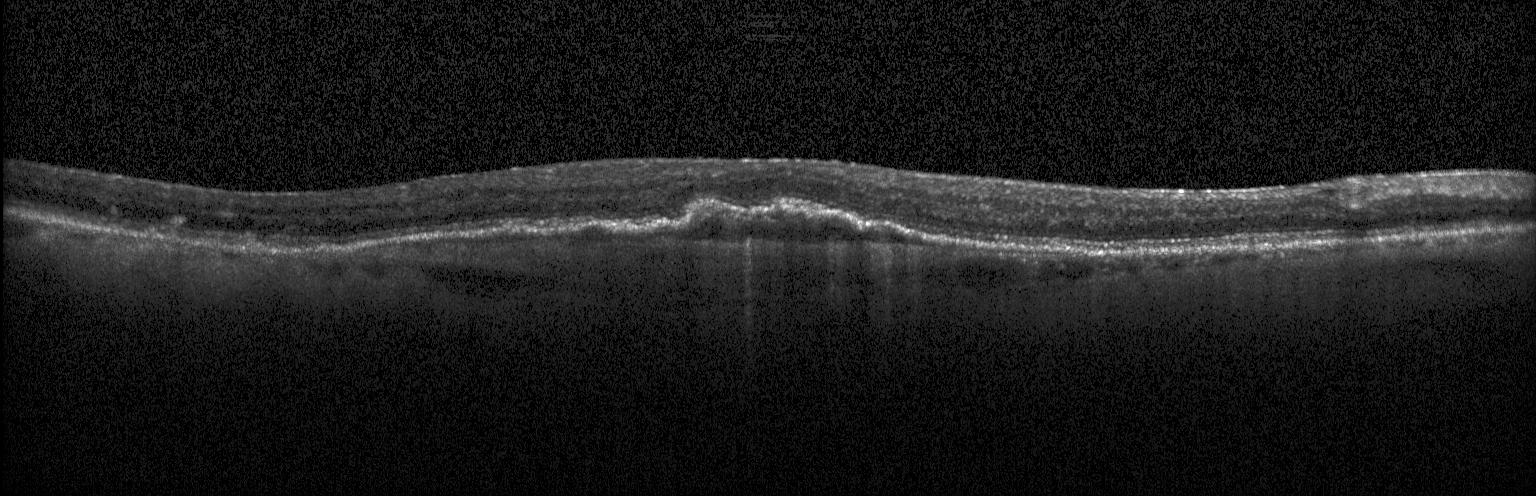 Impression: choroidal neovascularization.